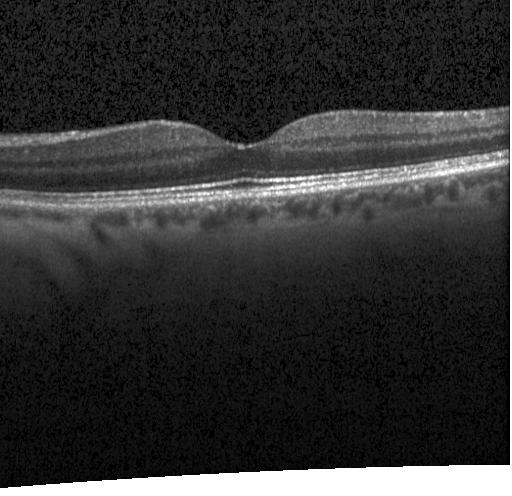 Macular OCT demonstrating no choroidal neovascularization, no diabetic macular edema, and no drusen.